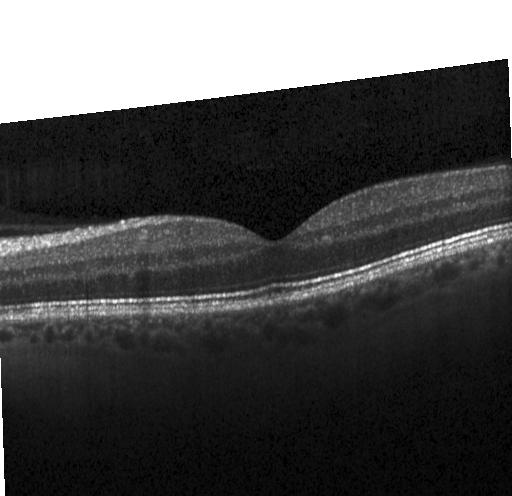

Acquired on a Heidelberg Spectralis · spectral-domain OCT · centered on the fovea · optical coherence tomography scan — Diagnosis: no CNV, DME, or drusen.